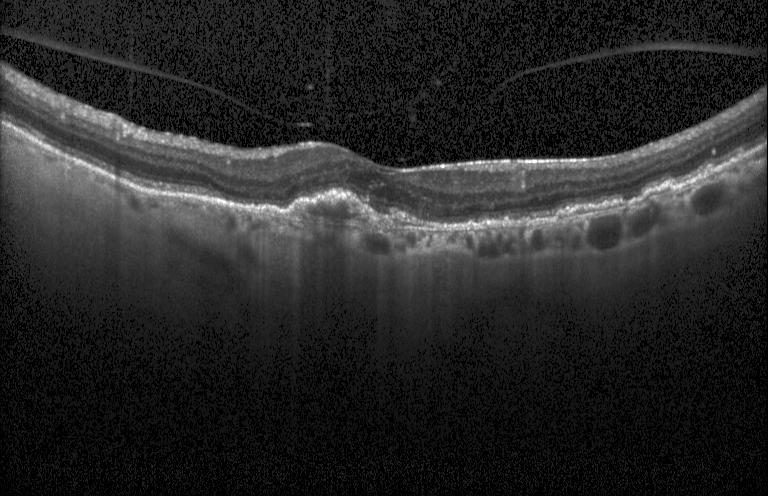

Retinal OCT cross-section — OCT finding: CNV.